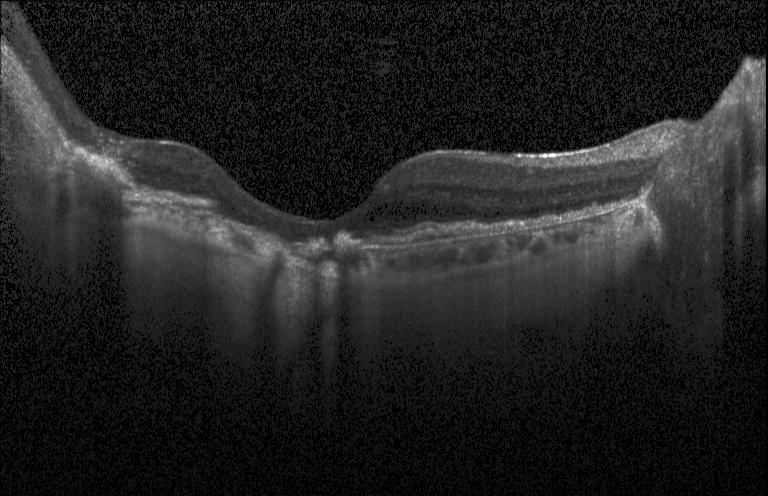
Acquired on a Heidelberg Spectralis · retinal OCT cross-section · spectral-domain OCT. This B-scan demonstrates a choroidal neovascular membrane.